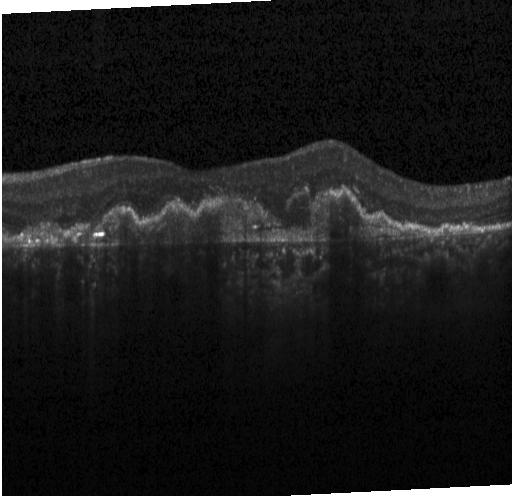

Spectral-domain optical coherence tomography · macular scan · acquired on a Heidelberg Spectralis · retinal OCT cross-section — Choroidal neovascularization.